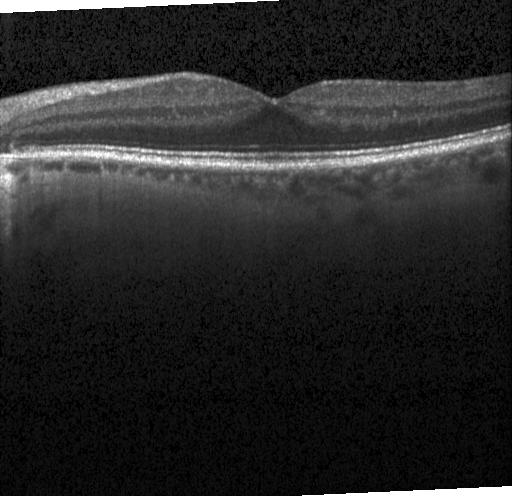 Instrument: Heidelberg Spectralis · macular scan · OCT B-scan · spectral-domain optical coherence tomography.
Dx: no choroidal neovascularization, no diabetic macular edema, and no drusen.